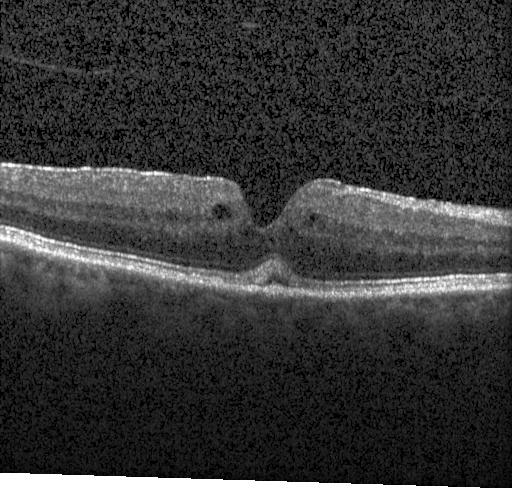
Acquired on a Heidelberg Spectralis, OCT B-scan, fovea-centered, spectral-domain OCT. Impression: DME.